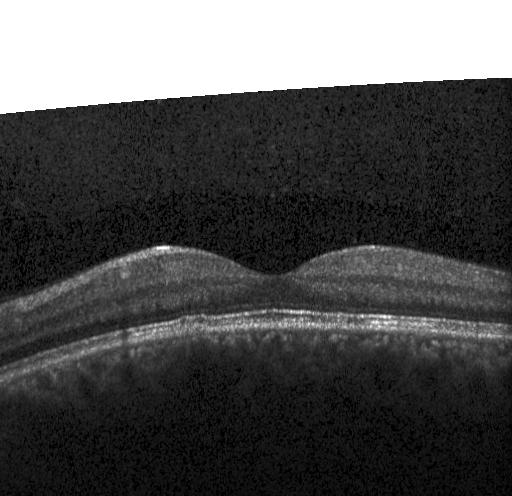
Macular scan, instrument: Heidelberg Spectralis, optical coherence tomography B-scan — Diagnosis: no CNV, DME, or drusen.